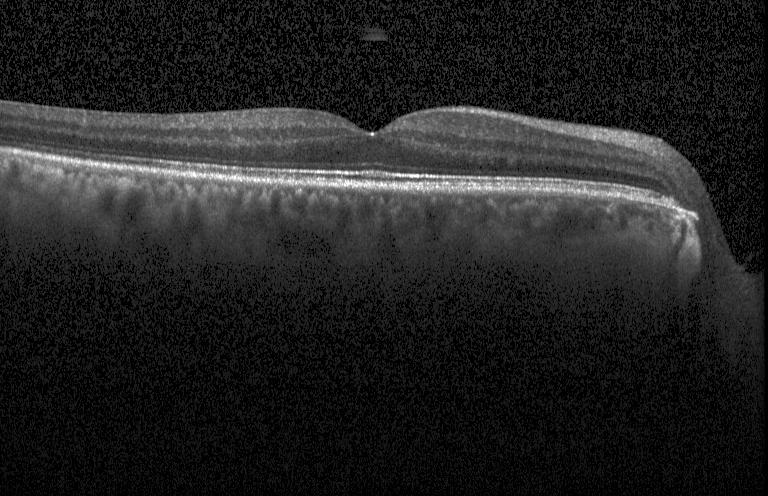 Dx: no choroidal neovascularization, no diabetic macular edema, and no drusen.